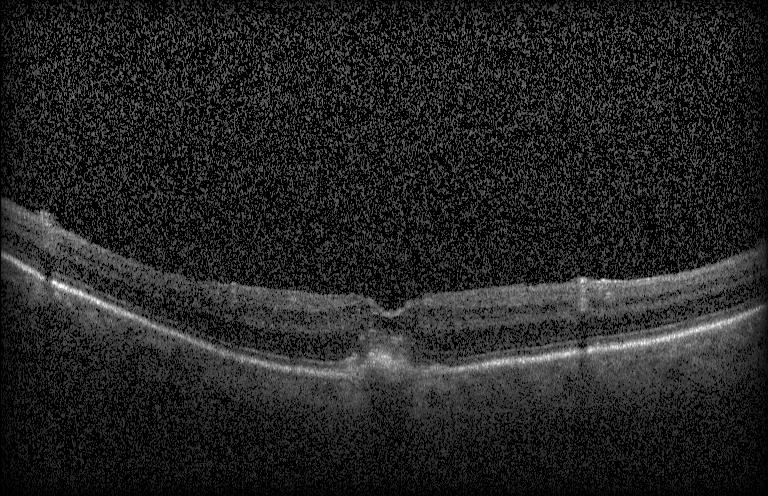 Heidelberg Spectralis. Spectral-domain optical coherence tomography. Retinal OCT cross-section — Diagnosis: a choroidal neovascular membrane.